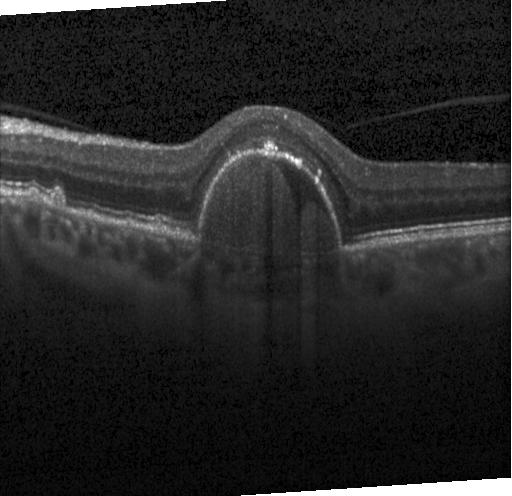
Macular OCT demonstrating a choroidal neovascular membrane.